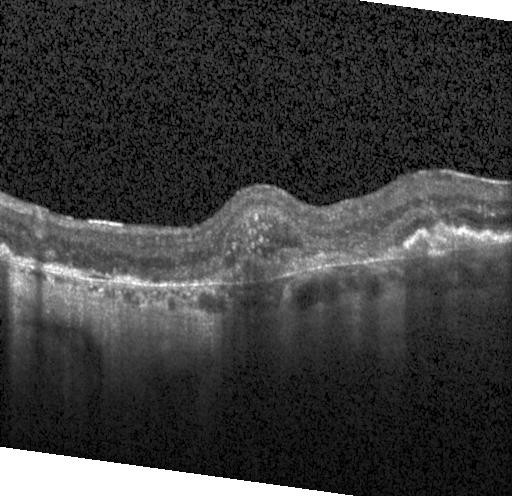
Finding: a choroidal neovascular membrane.